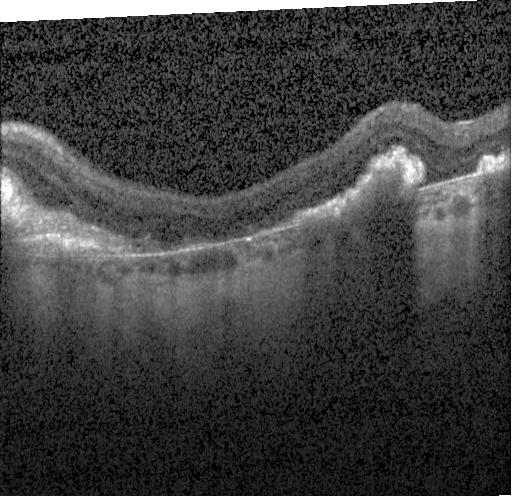 Retinal OCT cross-section; Heidelberg Spectralis.
A choroidal neovascular membrane.